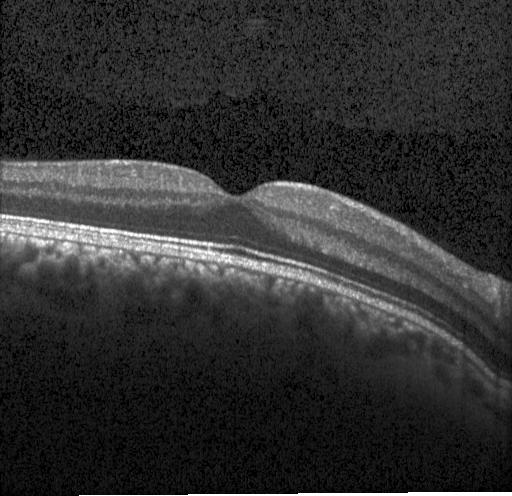 OCT line scan — Finding: neither choroidal neovascularization, diabetic macular edema, nor drusen.